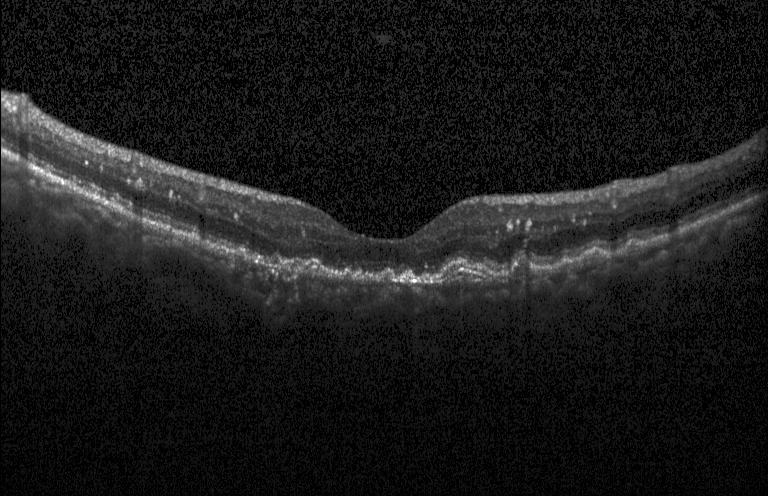 Retinal OCT cross-section; acquired on a Heidelberg Spectralis. Assessment: a choroidal neovascular membrane.